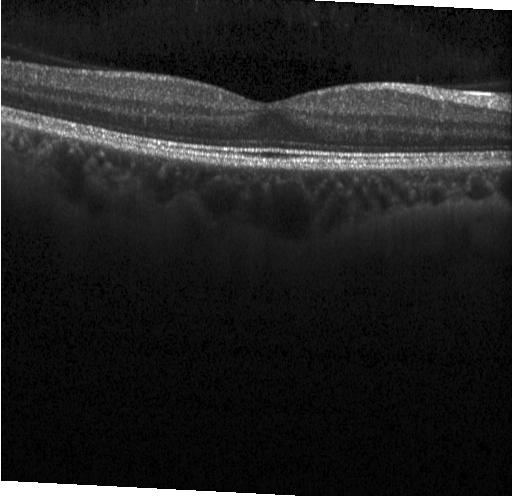

SD-OCT. OCT line scan.
Macular OCT: no CNV, DME, or drusen.